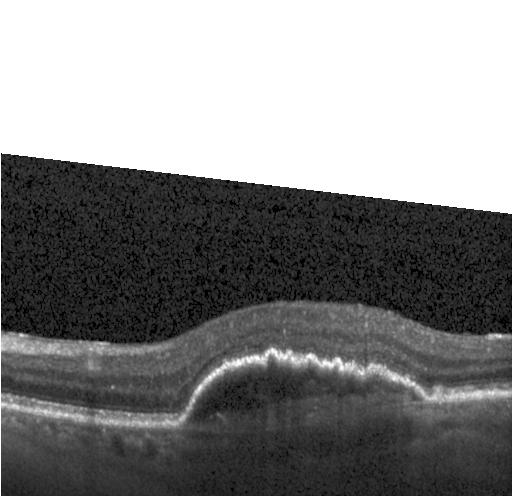
Macular OCT demonstrating CNV.